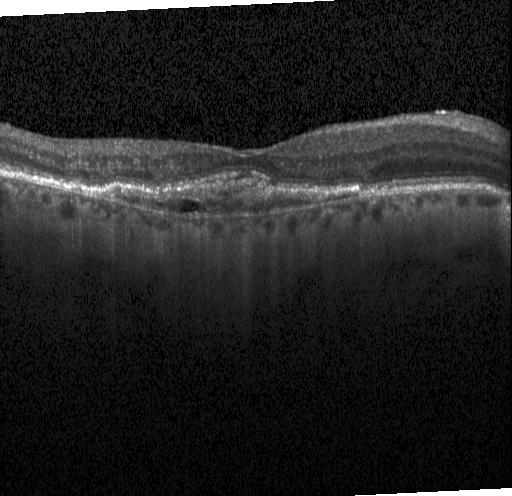

Diagnosis: choroidal neovascularization.